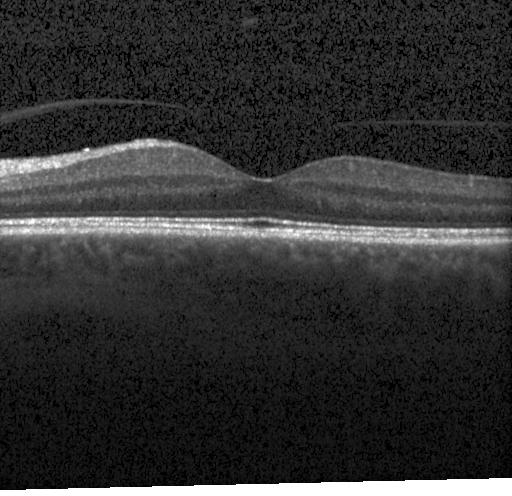
Heidelberg Spectralis OCT system, optical coherence tomography scan, spectral-domain OCT.
The scan shows no CNV, DME, or drusen.